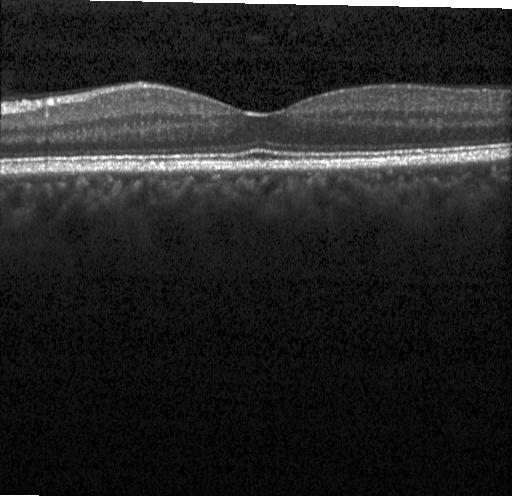 Heidelberg Spectralis. Macular scan. Optical coherence tomography scan.
Macular OCT: neither choroidal neovascularization, diabetic macular edema, nor drusen.